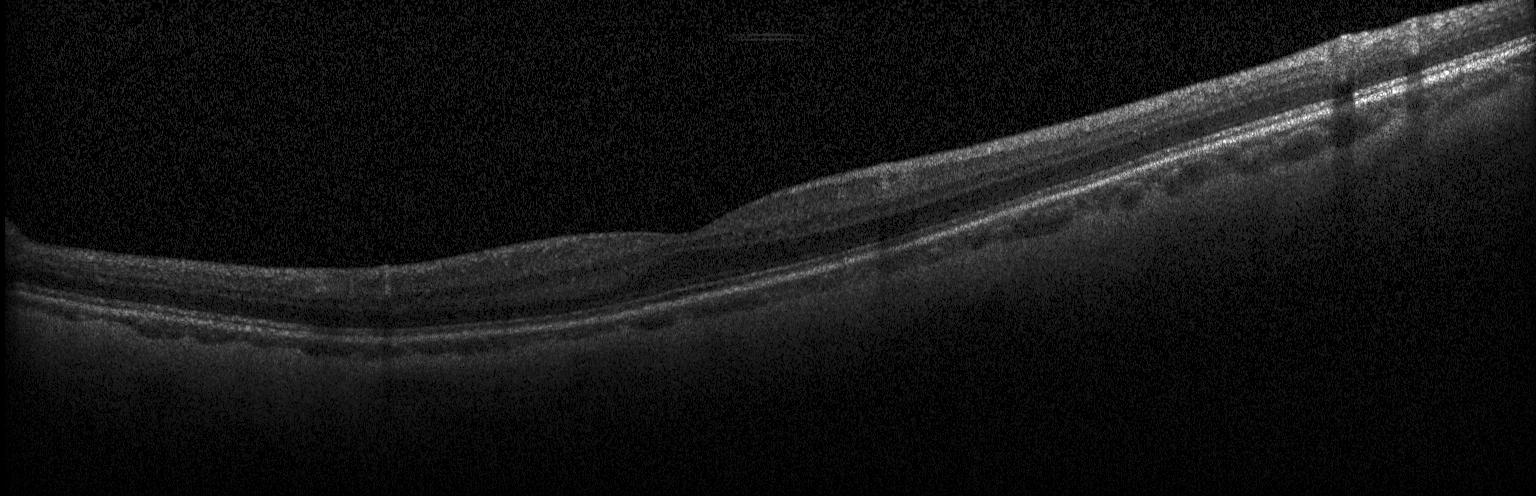
Neither choroidal neovascularization, diabetic macular edema, nor drusen.